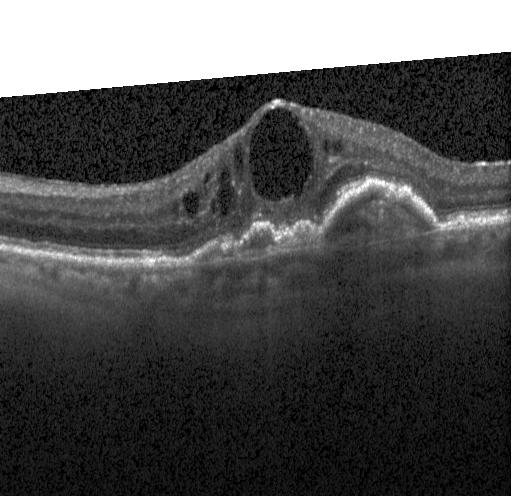 Macular OCT demonstrating choroidal neovascularization (CNV).